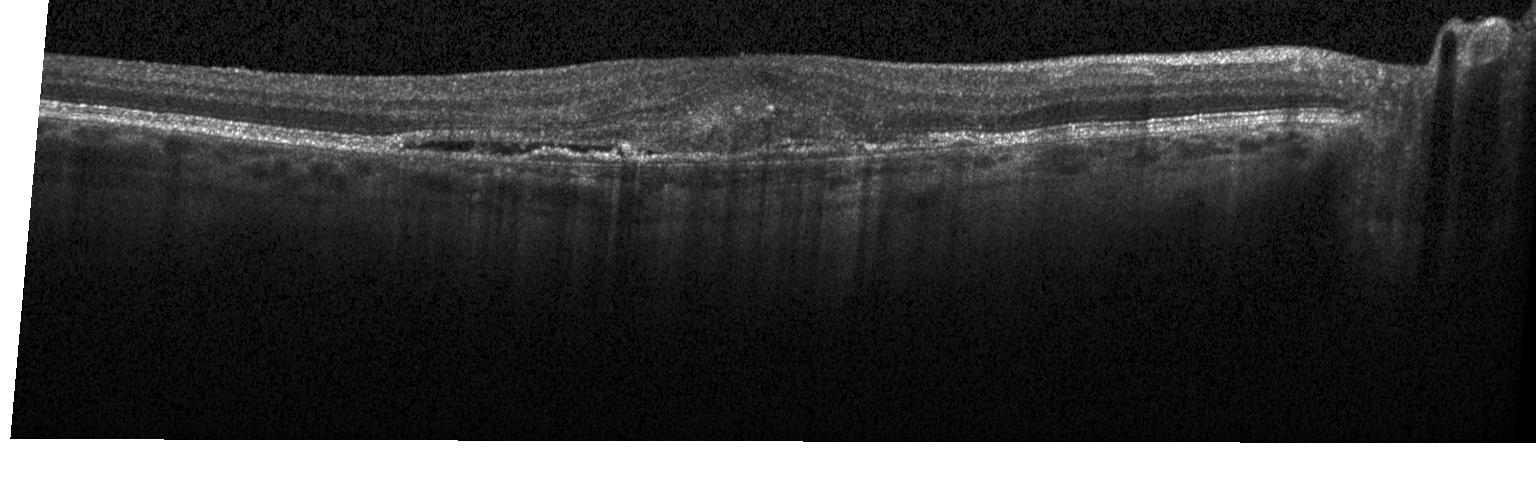
Impression: choroidal neovascularization (CNV).